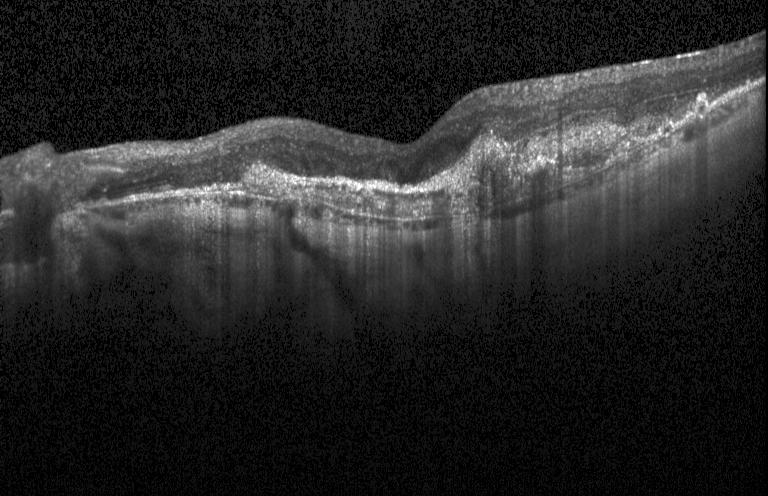
Acquired on a Heidelberg Spectralis; optical coherence tomography B-scan; spectral-domain OCT; fovea-centered.
Impression: choroidal neovascularization (CNV).